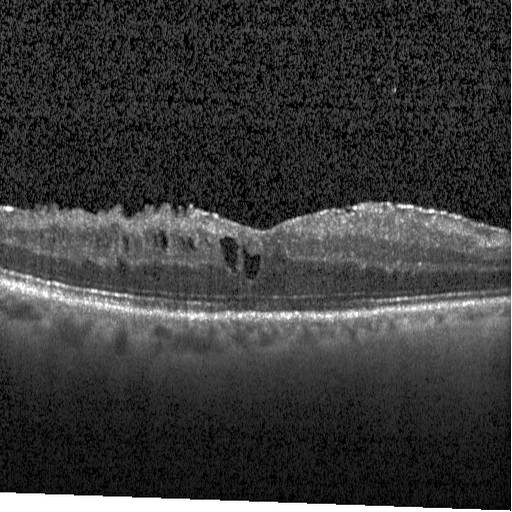 OCT finding: diabetic macular edema (DME).